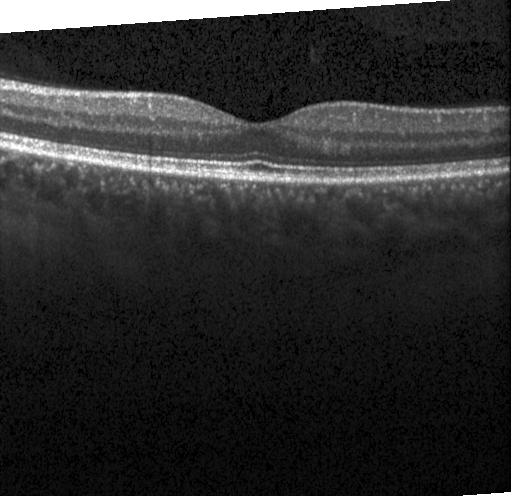
Retinal OCT B-scan. SD-OCT. Macular scan. The scan shows no evidence of CNV, DME, or drusen.